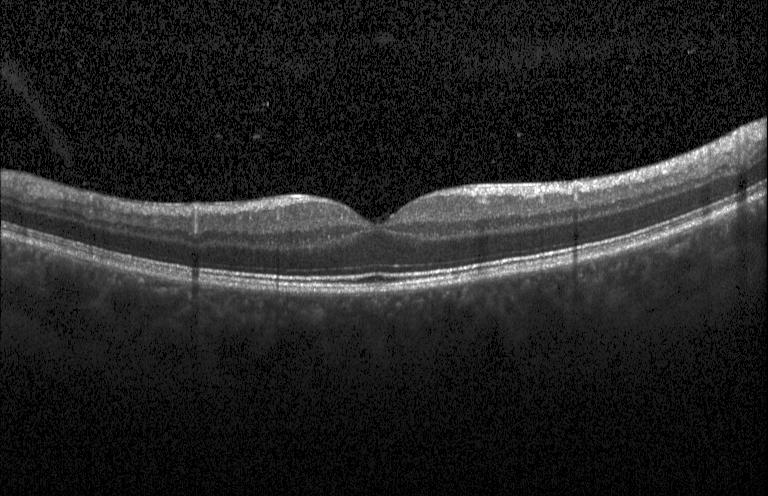 Optical coherence tomography scan
Diagnosis: no evidence of CNV, DME, or drusen.